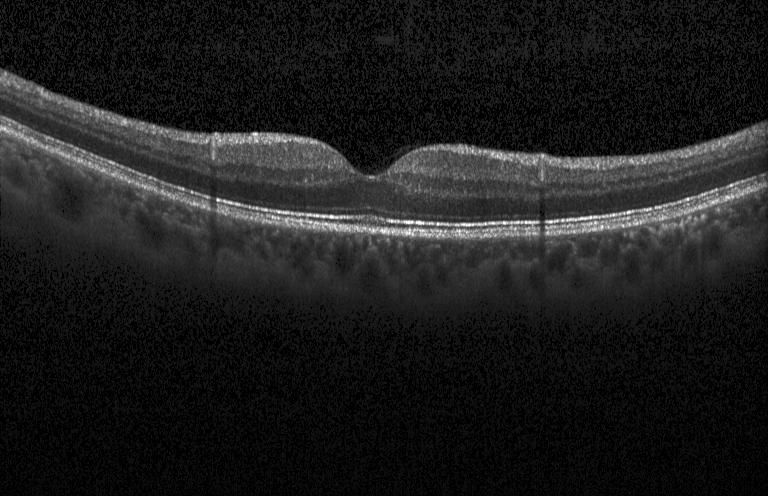
Neither choroidal neovascularization, diabetic macular edema, nor drusen.